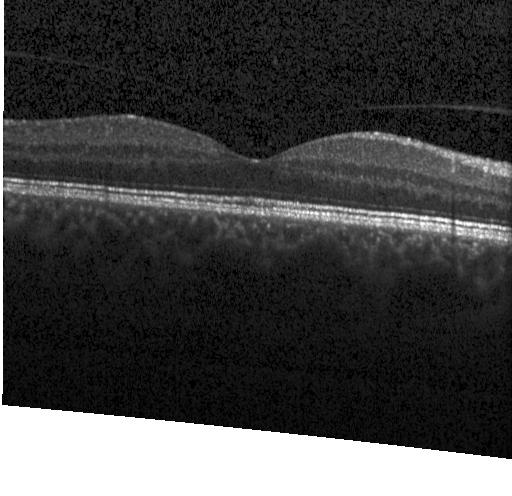

OCT B-scan showing neither choroidal neovascularization, diabetic macular edema, nor drusen.